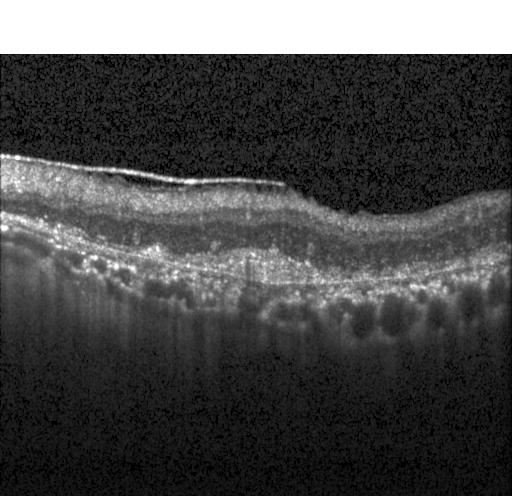

Spectral-domain OCT B-scan: a choroidal neovascular membrane.